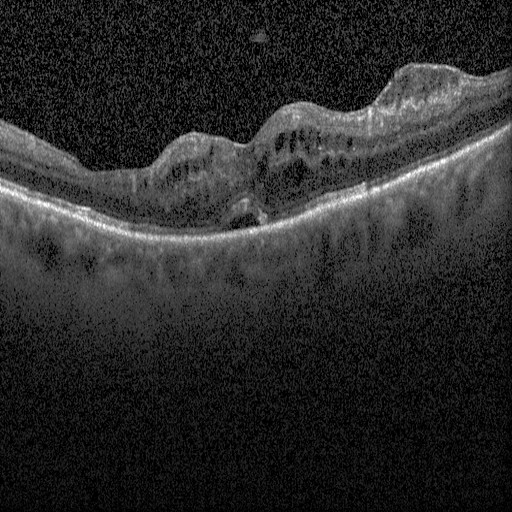
The scan shows diabetic macular edema (DME).